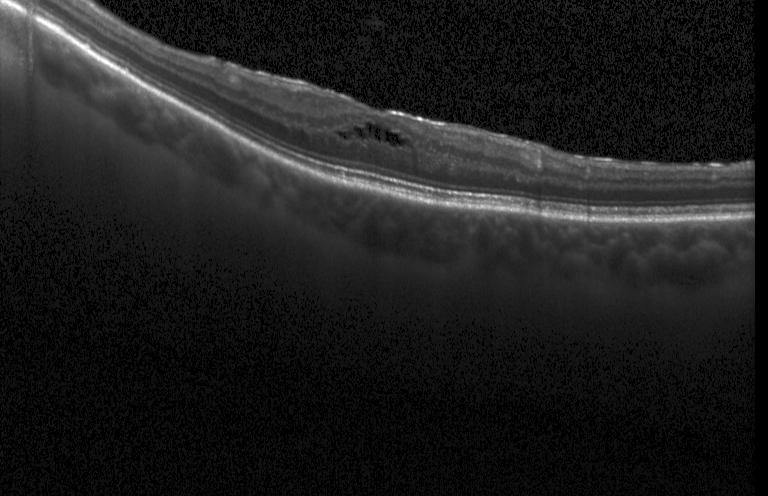
Retinal OCT B-scan · spectral-domain OCT · instrument: Heidelberg Spectralis.
Macular OCT: diabetic macular edema.